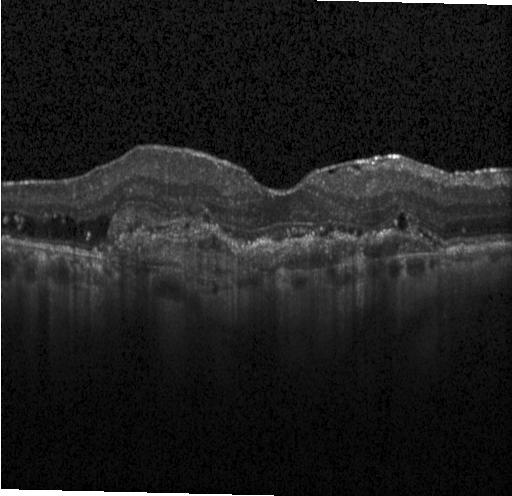 Horizontal scan through the fovea, retinal OCT cross-section, spectral-domain OCT — OCT finding: CNV.